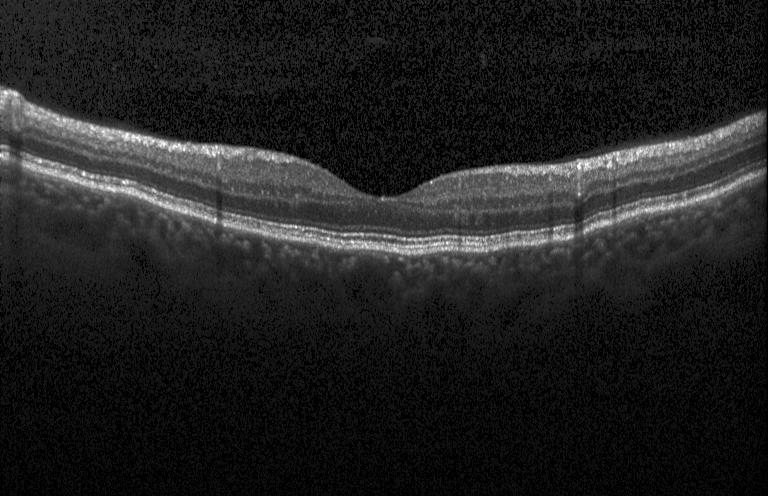

OCT line scan
Finding: no choroidal neovascularization, no diabetic macular edema, and no drusen.